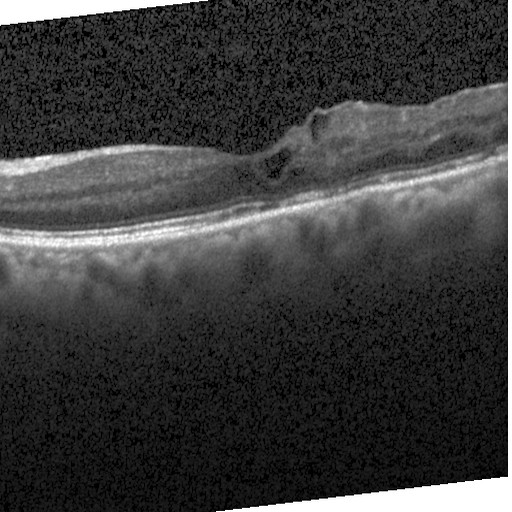 Horizontal scan through the fovea · acquired on a Heidelberg Spectralis · SD-OCT · OCT B-scan. This B-scan demonstrates diabetic macular edema.